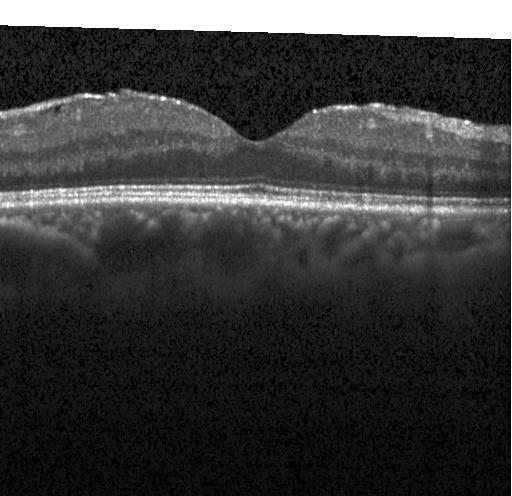

OCT finding: no evidence of CNV, DME, or drusen.